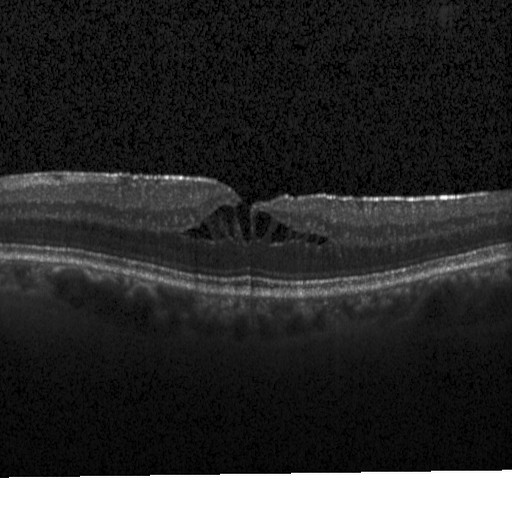

Assessment: DME.